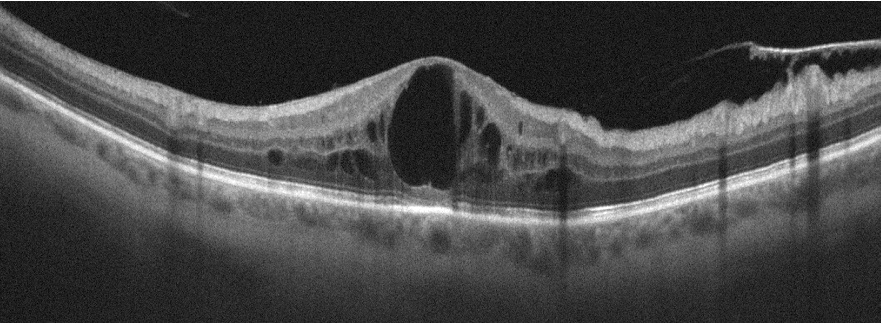
Optical coherence tomography scan · Optovue Avanti RTVue XR — Diagnosis: diabetic macular edema.